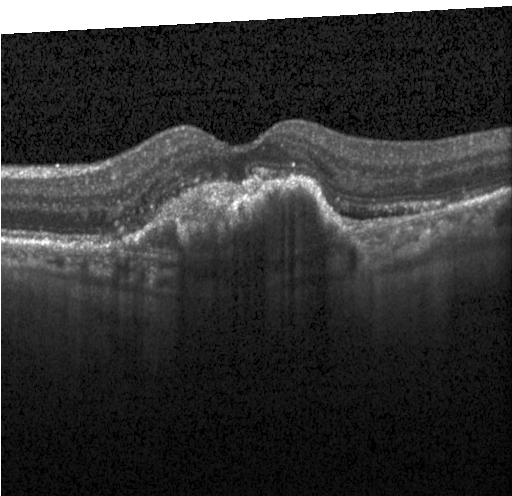
The scan shows a choroidal neovascular membrane.